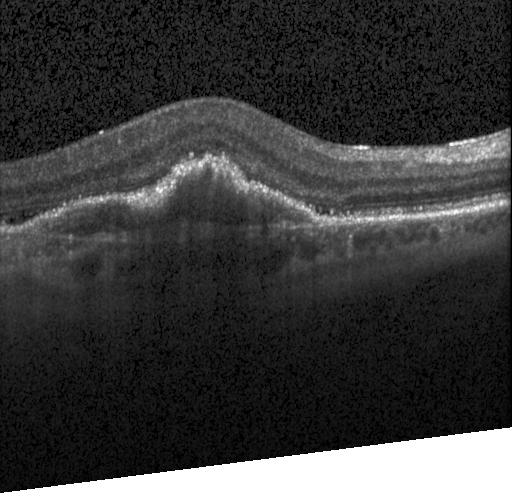 Instrument: Heidelberg Spectralis · optical coherence tomography B-scan
Finding: choroidal neovascularization (CNV).